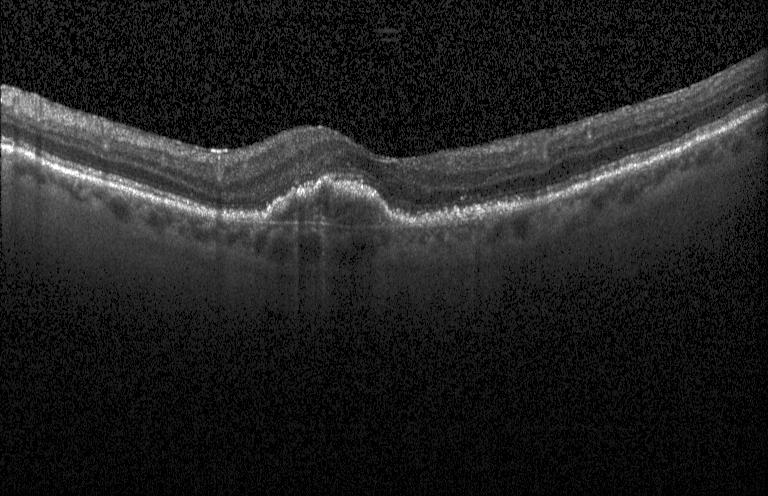

OCT B-scan
Impression: a choroidal neovascular membrane.